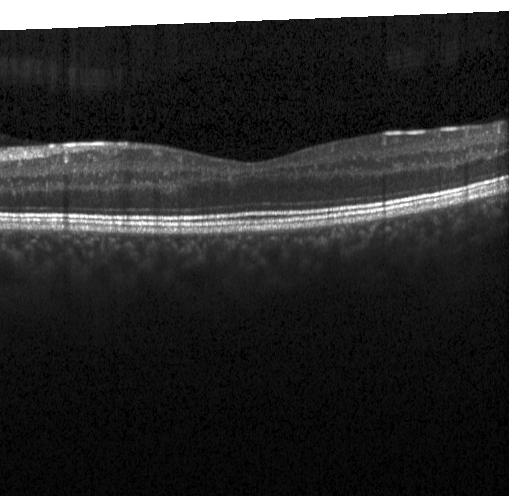 Optical coherence tomography B-scan.
Neither choroidal neovascularization, diabetic macular edema, nor drusen.